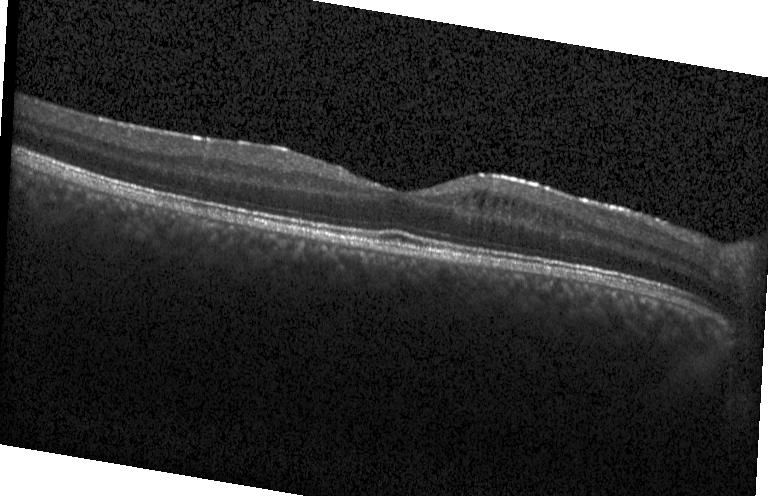

Spectral-domain optical coherence tomography; optical coherence tomography B-scan
Impression: diabetic macular edema.